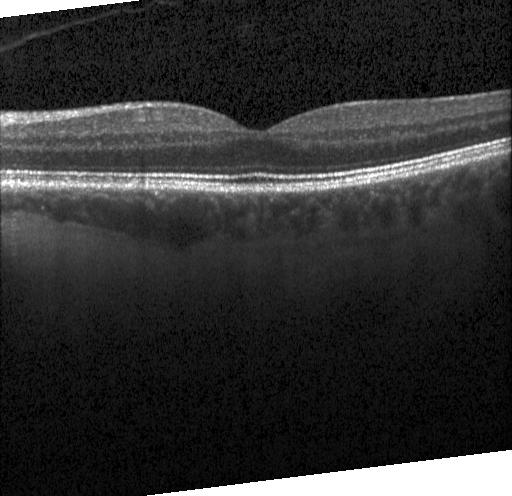
Assessment: no evidence of choroidal neovascularization, diabetic macular edema, or drusen.